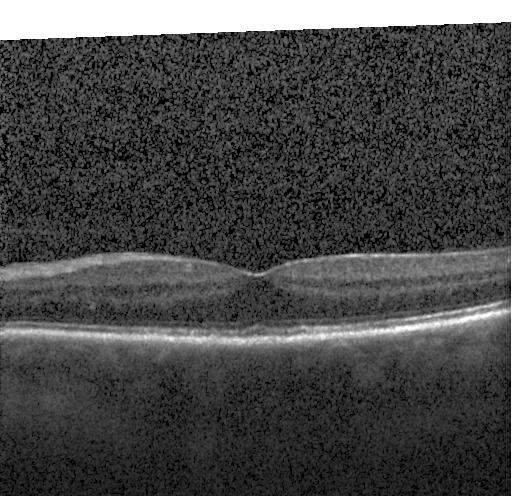
Finding: no CNV, DME, or drusen.